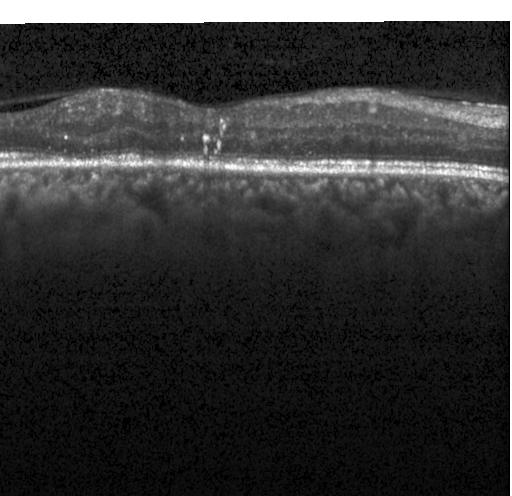

Optical coherence tomography B-scan · through the macula. The scan shows diabetic macular edema (DME).